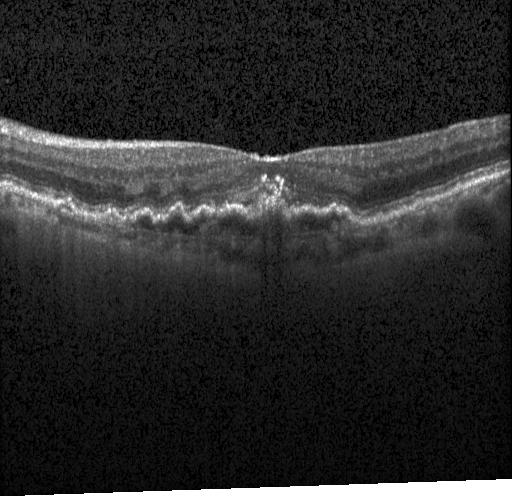
OCT line scan. Impression: choroidal neovascularization.